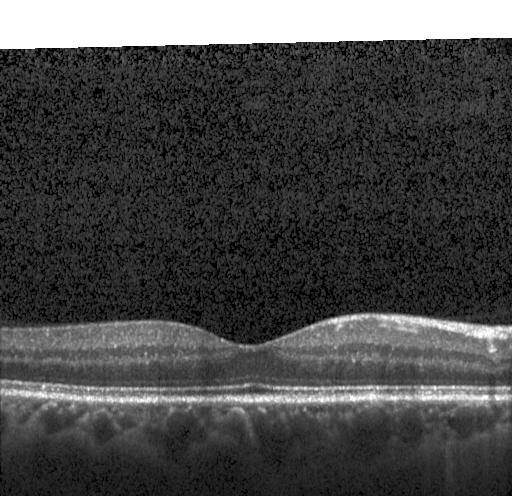

Dx: no evidence of choroidal neovascularization, diabetic macular edema, or drusen.